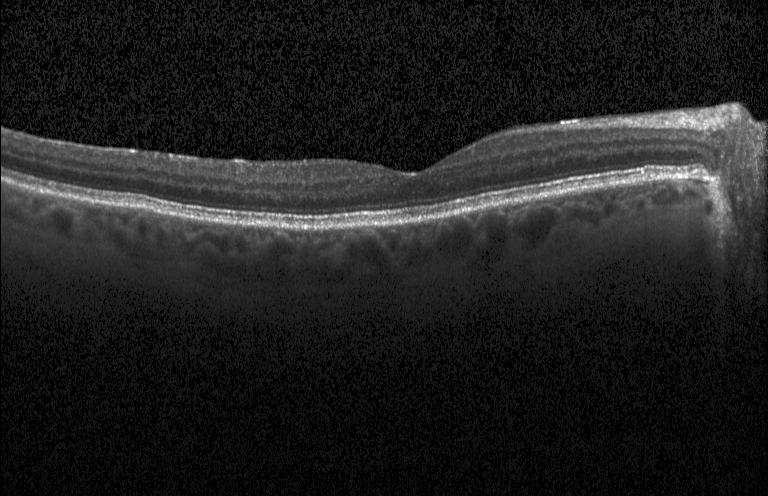

Finding: no CNV, no DME, and no drusen.